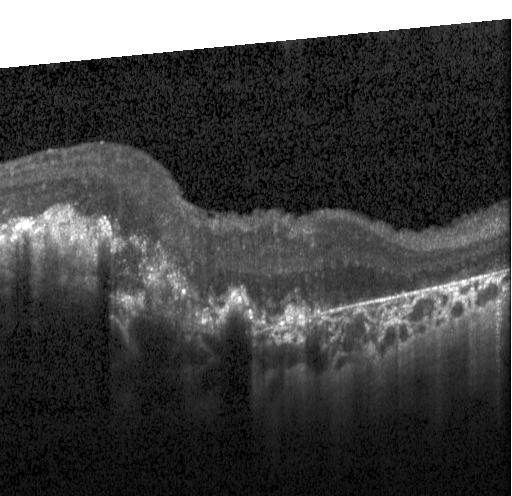
Finding: a choroidal neovascular membrane.